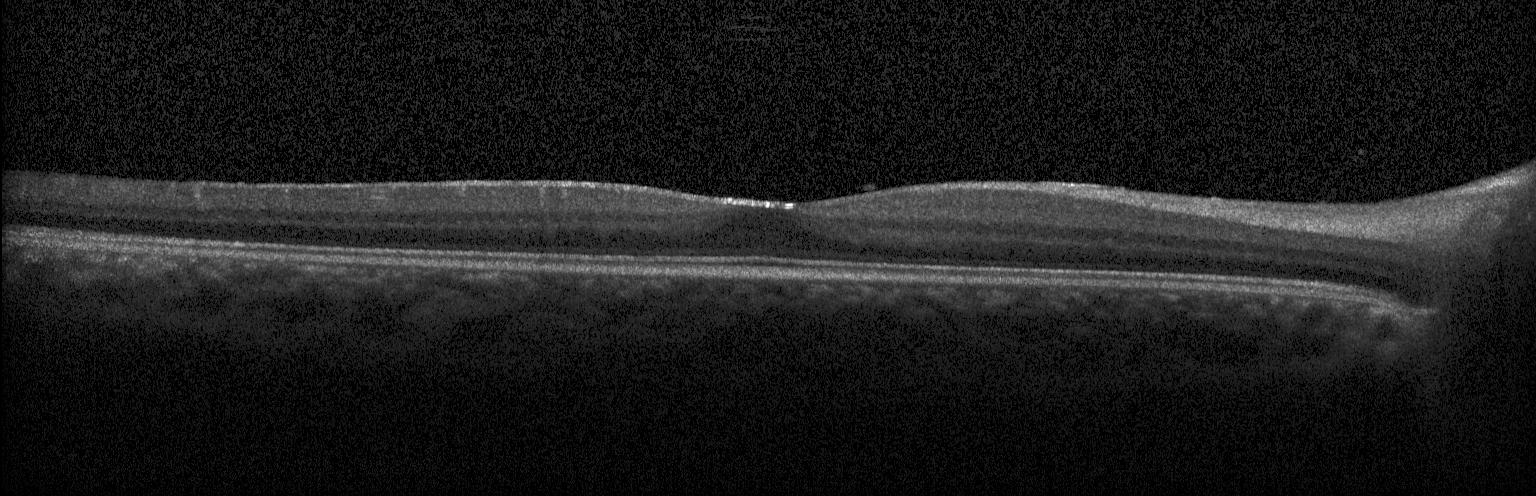
The scan shows no CNV, no DME, and no drusen.